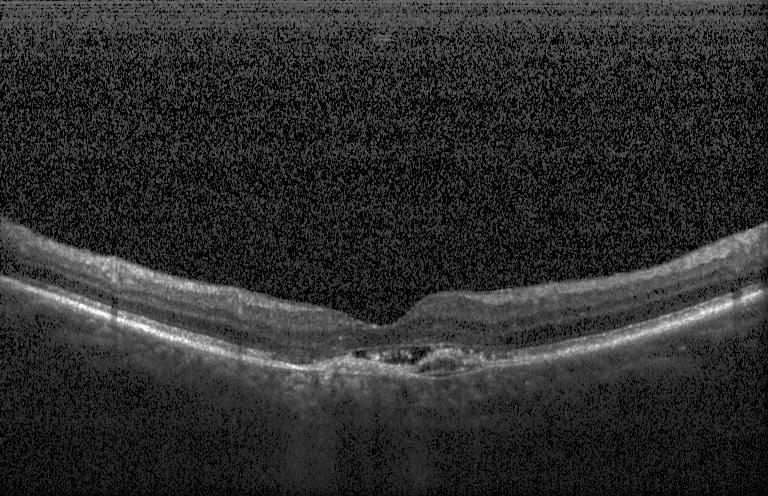

Optical coherence tomography scan; spectral-domain optical coherence tomography; centered on the fovea; acquired on a Heidelberg Spectralis
Assessment: a choroidal neovascular membrane.